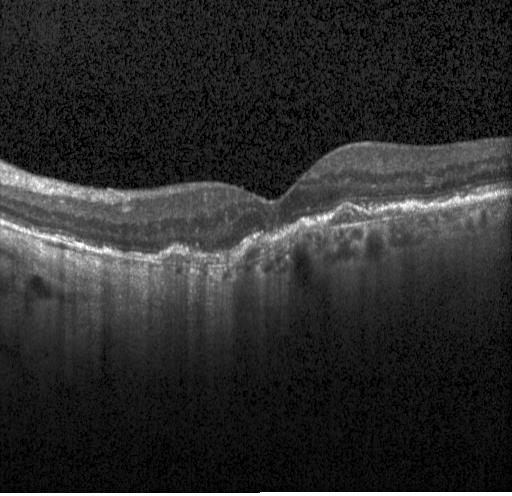 Retinal OCT B-scan — OCT finding: a choroidal neovascular membrane.